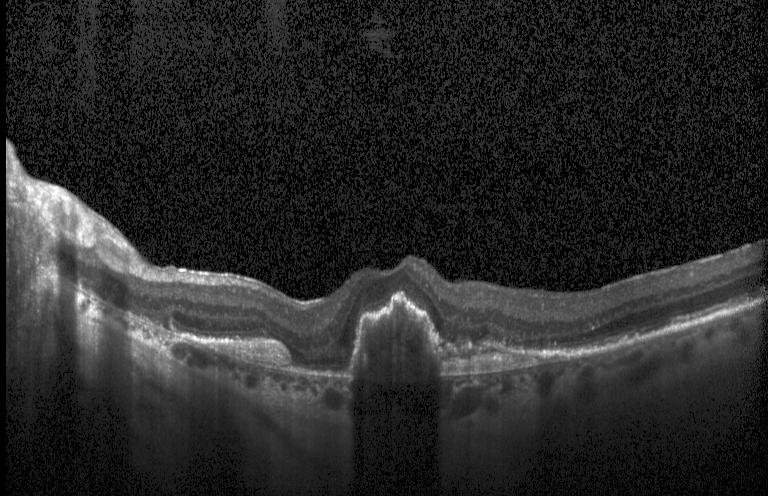 This B-scan demonstrates a choroidal neovascular membrane.